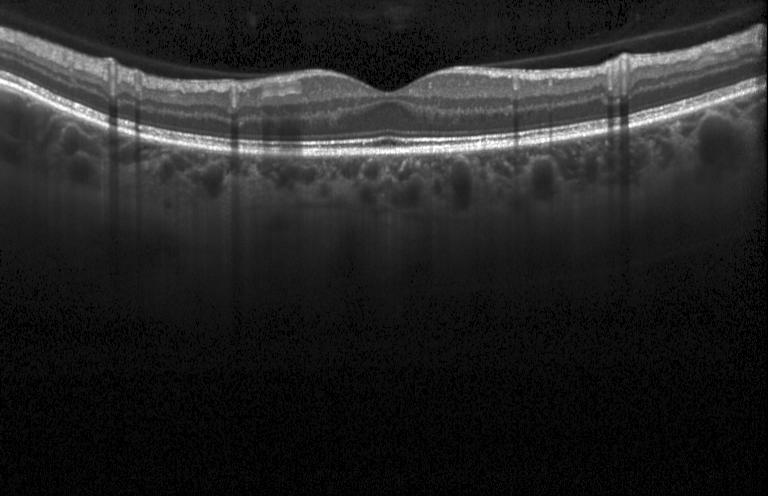
Instrument: Heidelberg Spectralis · horizontal scan through the fovea · spectral-domain OCT · retinal OCT B-scan.
The scan shows neither choroidal neovascularization, diabetic macular edema, nor drusen.